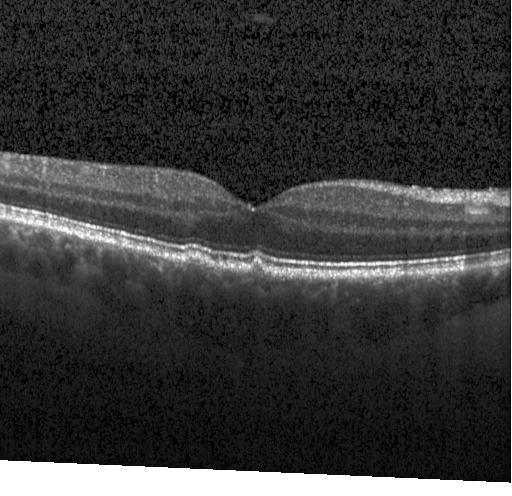 Impression: drusen.